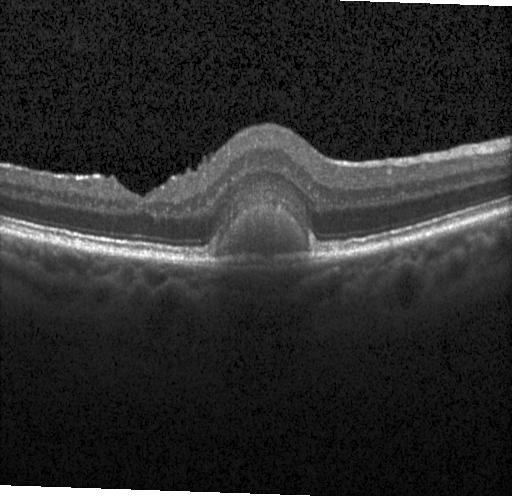 Macular OCT: choroidal neovascularization (CNV).